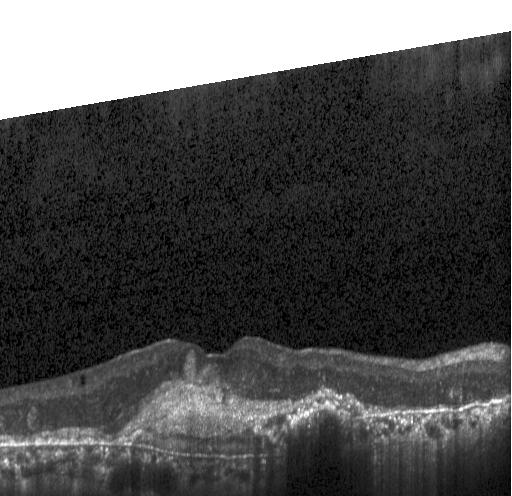

OCT B-scan. This B-scan demonstrates choroidal neovascularization (CNV).